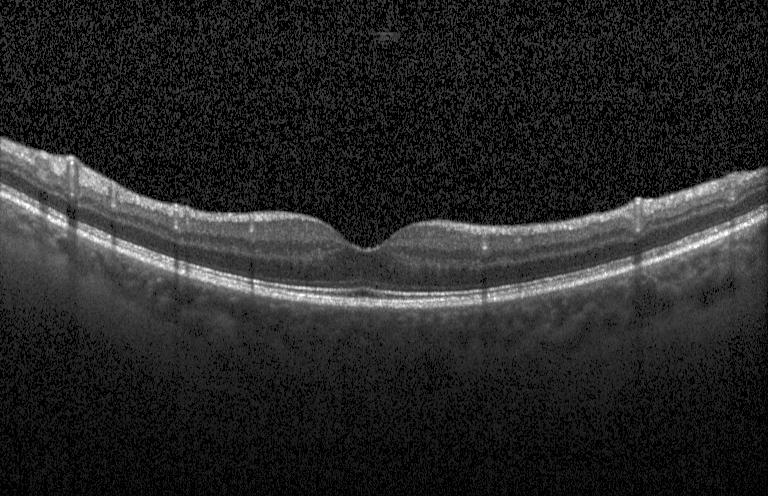

Optical coherence tomography B-scan, acquired on a Heidelberg Spectralis
Diagnosis: no choroidal neovascularization, no diabetic macular edema, and no drusen.